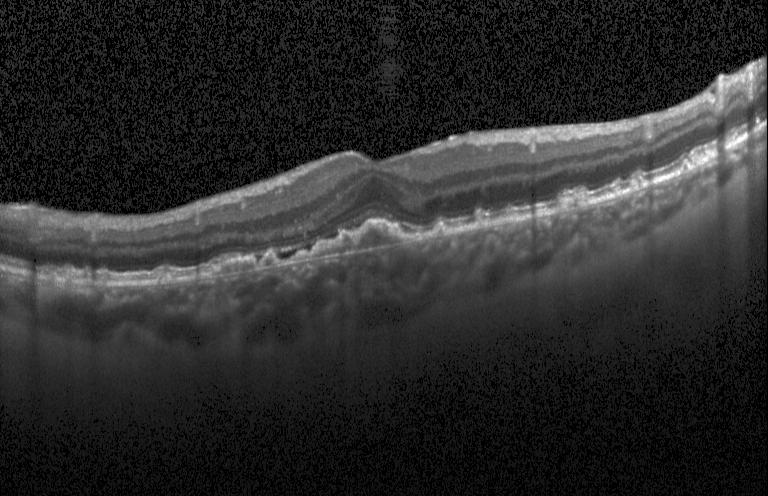

OCT finding: a choroidal neovascular membrane.